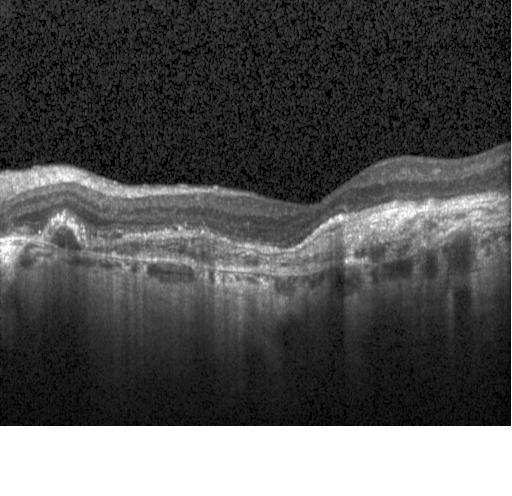 Centered on the fovea · spectral-domain optical coherence tomography · OCT line scan — The scan shows choroidal neovascularization (CNV).